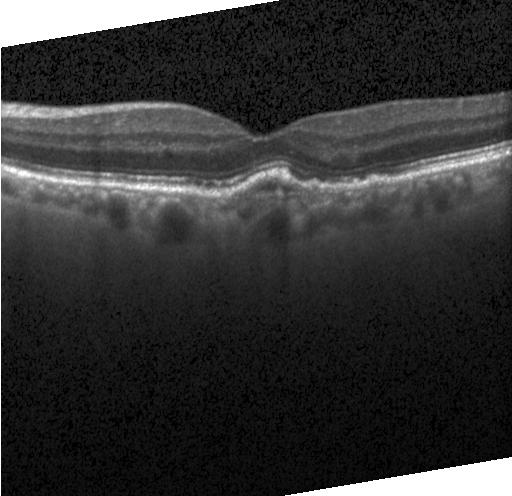

Macular OCT demonstrating CNV.